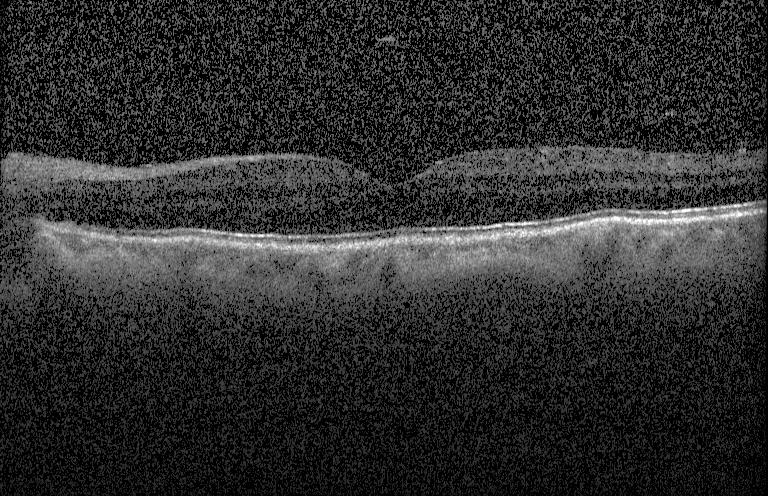
Spectral-domain OCT · OCT B-scan. This B-scan demonstrates neither choroidal neovascularization, diabetic macular edema, nor drusen.